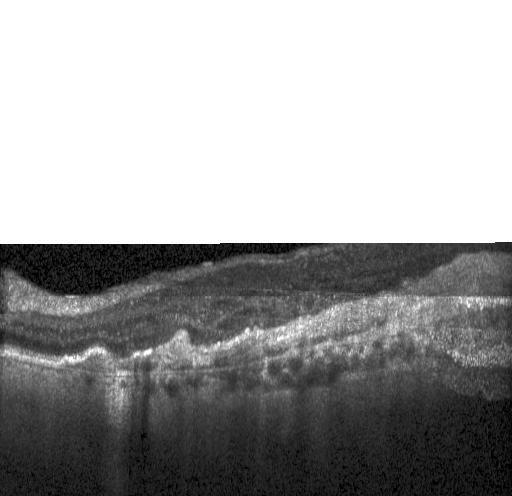

Retinal OCT cross-section. Spectral-domain OCT.
Assessment: CNV.